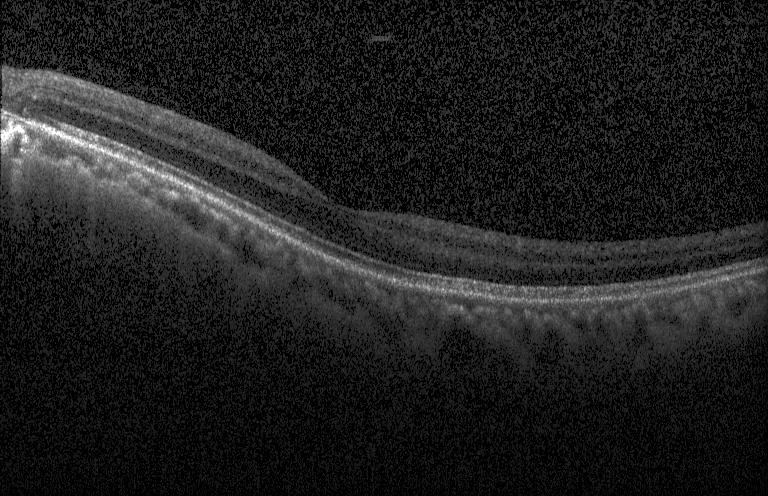

Heidelberg Spectralis · centered on the fovea · SD-OCT · OCT line scan
OCT finding: no evidence of CNV, DME, or drusen.